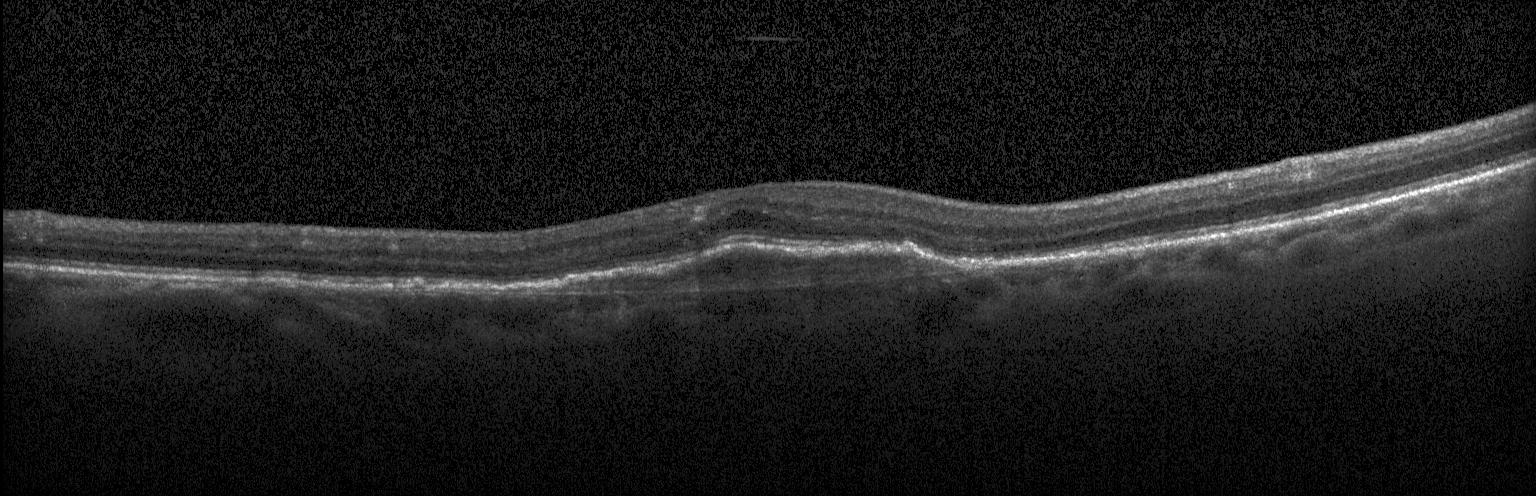 Macular OCT: a choroidal neovascular membrane.